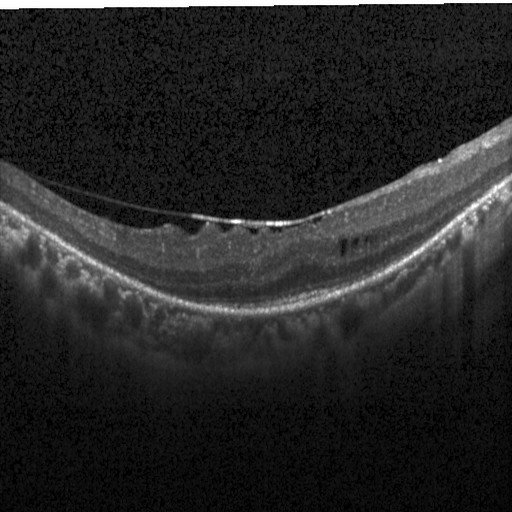
Diagnosis: DME.